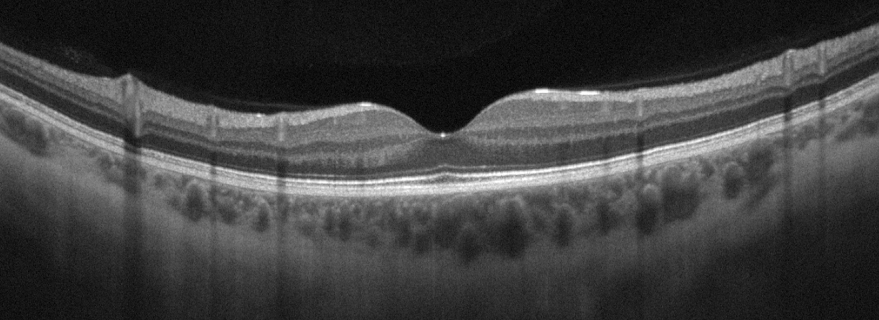

OCT line scan, through the macula.
Diagnosis: no AMD, DME, ERM, RAO, RVO, or VID.